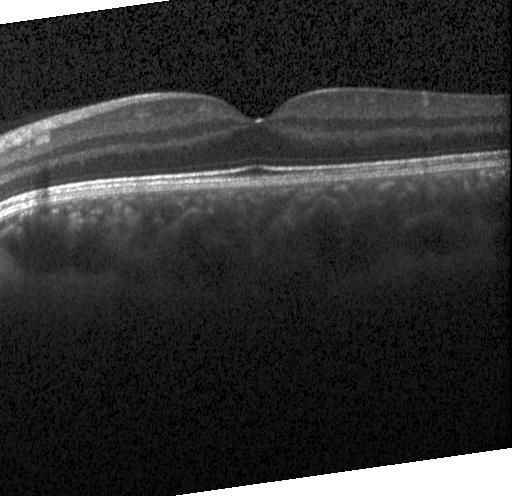
Dx: neither choroidal neovascularization, diabetic macular edema, nor drusen.